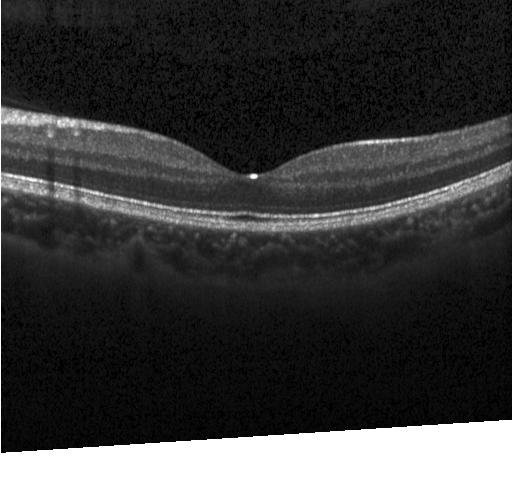

Diagnosis: no evidence of choroidal neovascularization, diabetic macular edema, or drusen.